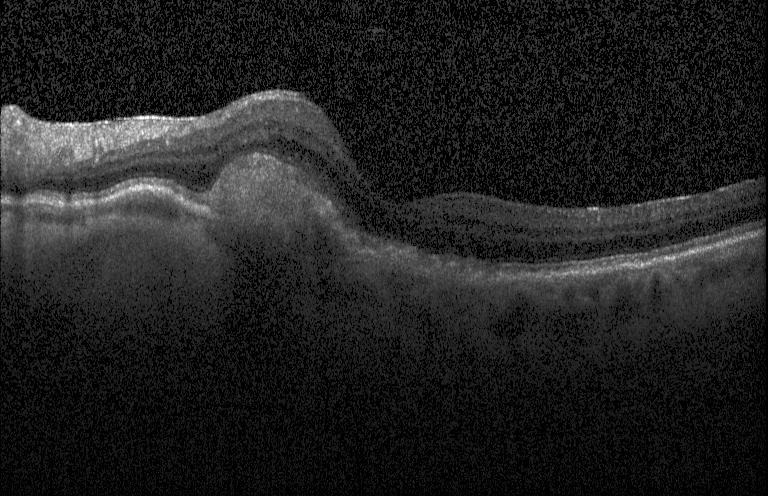 Impression: CNV.